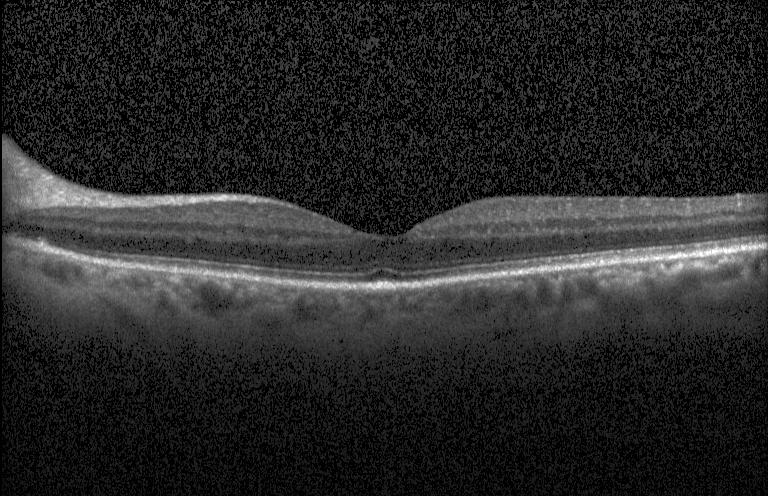 OCT finding: no evidence of choroidal neovascularization, diabetic macular edema, or drusen.